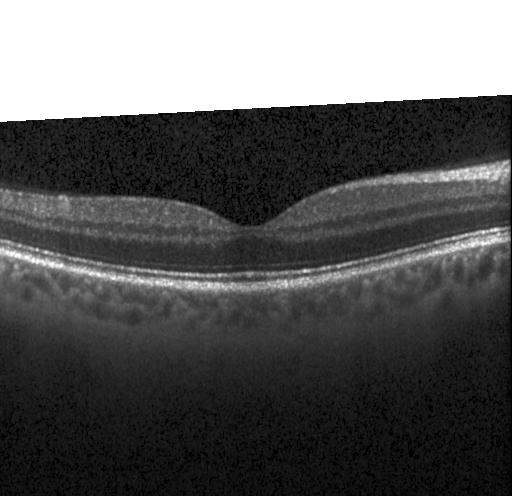 Optical coherence tomography B-scan.
Finding: no choroidal neovascularization, no diabetic macular edema, and no drusen.